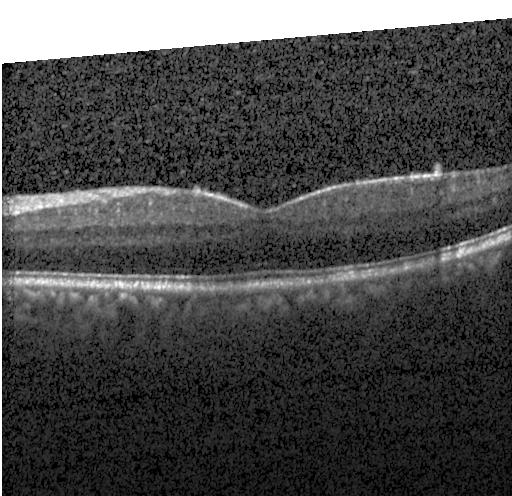
Spectral-domain OCT B-scan: no choroidal neovascularization, no diabetic macular edema, and no drusen.